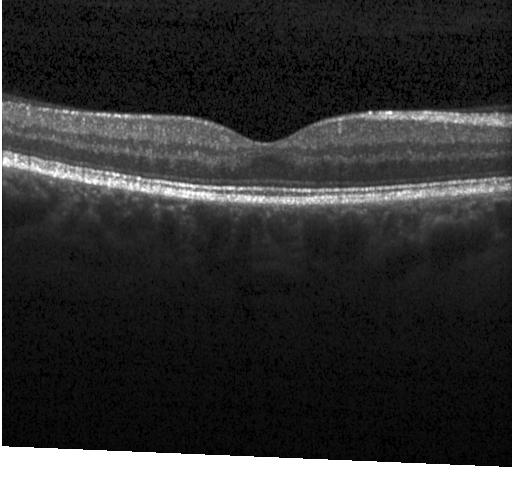

Optical coherence tomography scan · Heidelberg Spectralis OCT system.
Diagnosis: no choroidal neovascularization, diabetic macular edema, or drusen.